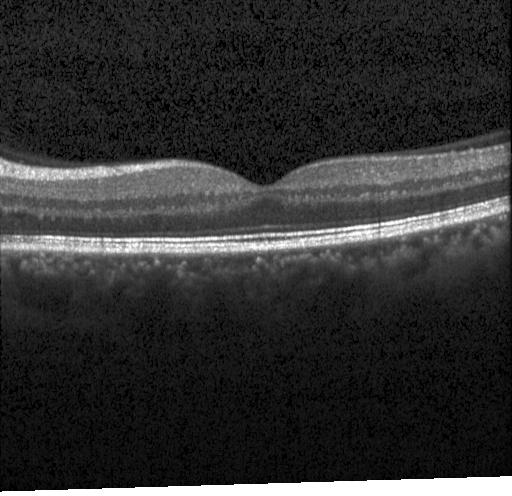

Optical coherence tomography B-scan. Impression: no choroidal neovascularization, diabetic macular edema, or drusen.